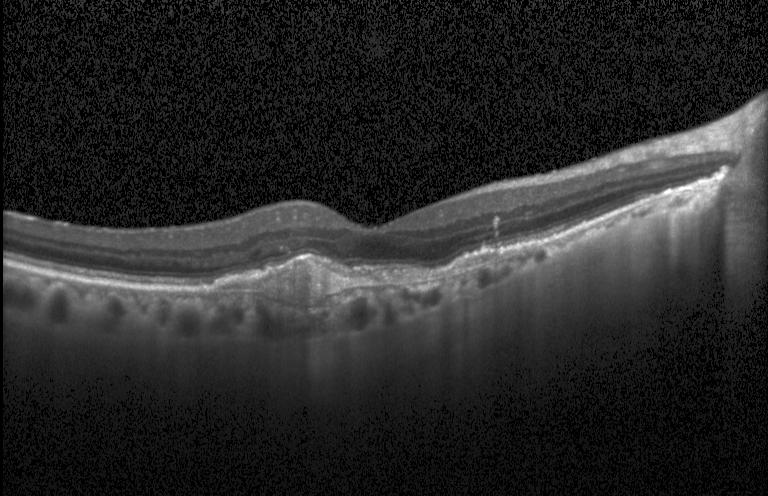 Instrument: Heidelberg Spectralis. Spectral-domain optical coherence tomography. Retinal OCT cross-section — Assessment: a choroidal neovascular membrane.